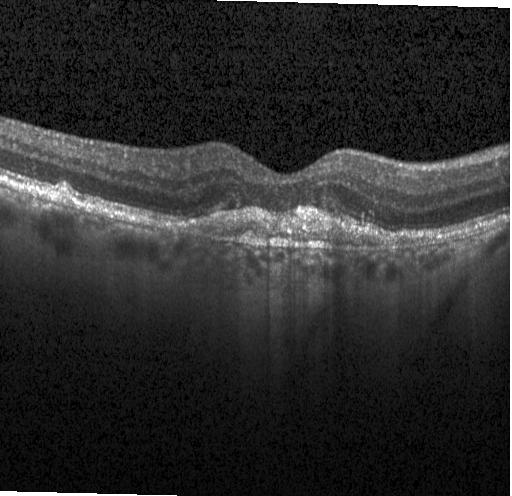 OCT line scan; horizontal scan through the fovea
Macular OCT: choroidal neovascularization.